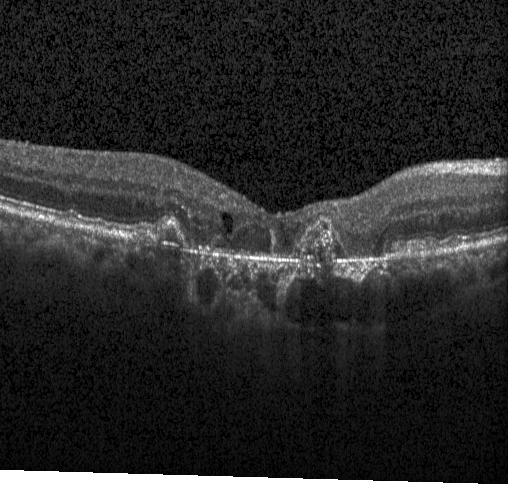 Diagnosis: a choroidal neovascular membrane.